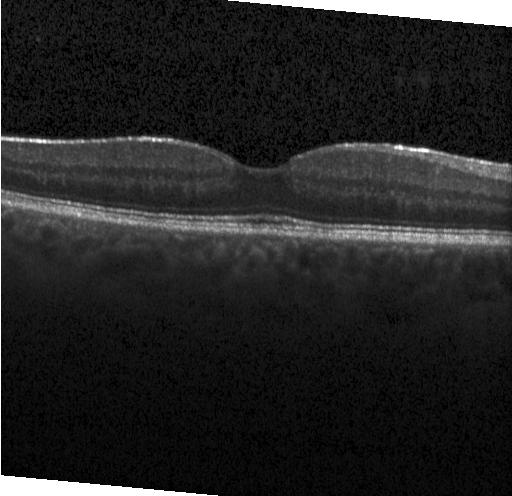
Finding: no CNV, DME, or drusen.